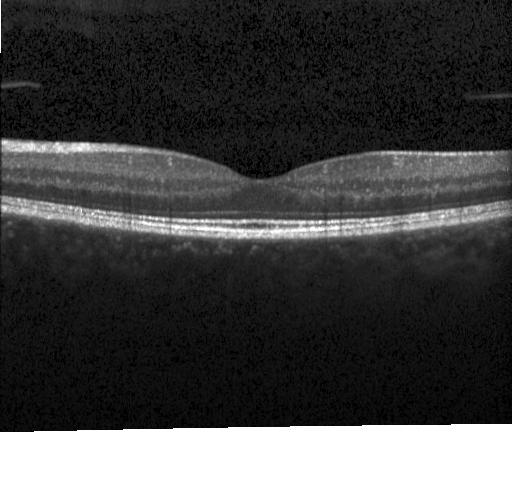
Spectral-domain OCT. OCT line scan. Through the macula. Heidelberg Spectralis OCT system. Diagnosis: no evidence of choroidal neovascularization, diabetic macular edema, or drusen.